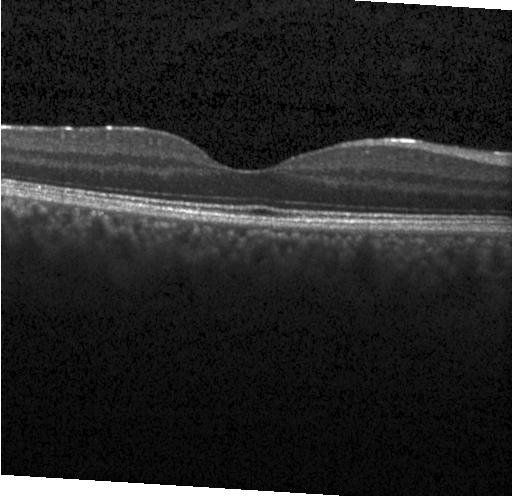

The scan shows no evidence of choroidal neovascularization, diabetic macular edema, or drusen.